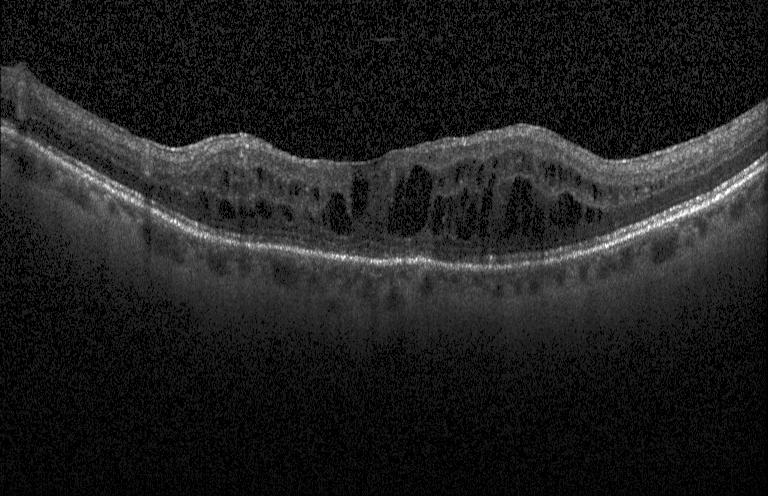

Fovea-centered. SD-OCT. Heidelberg Spectralis. OCT B-scan. Finding: diabetic macular edema (DME).